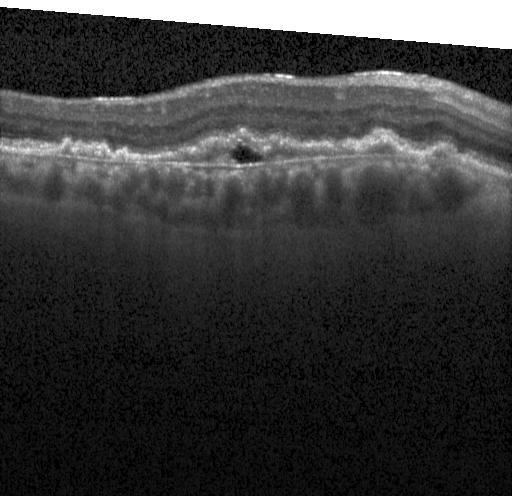

OCT B-scan, macular scan
Finding: a choroidal neovascular membrane.